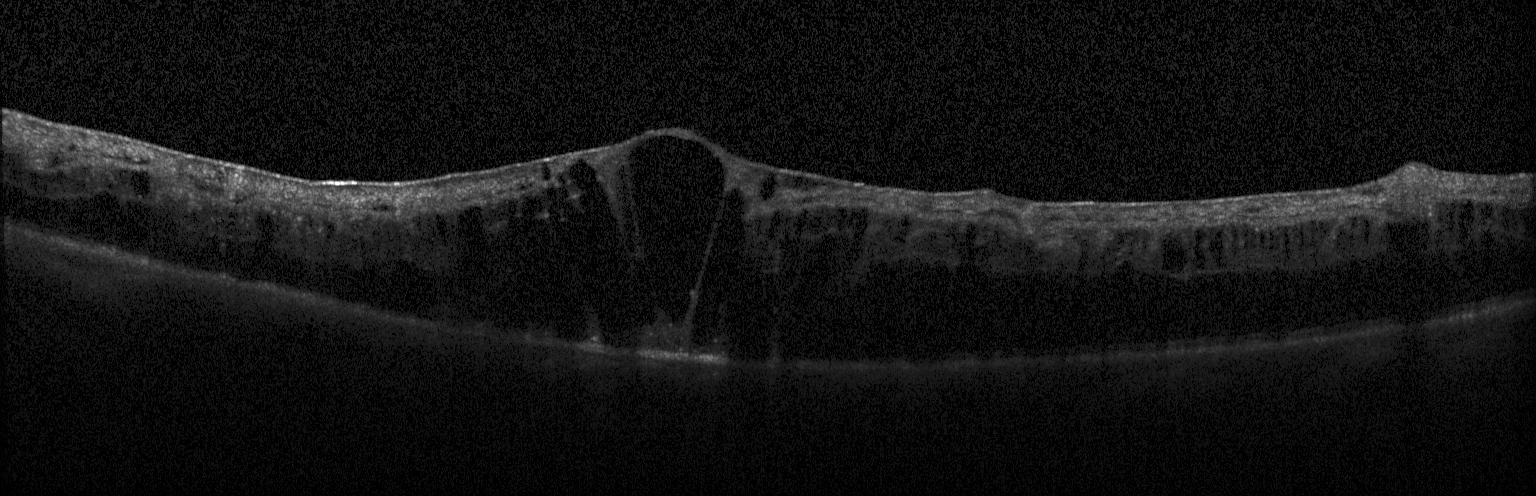 Heidelberg Spectralis. OCT line scan.
Impression: DME.